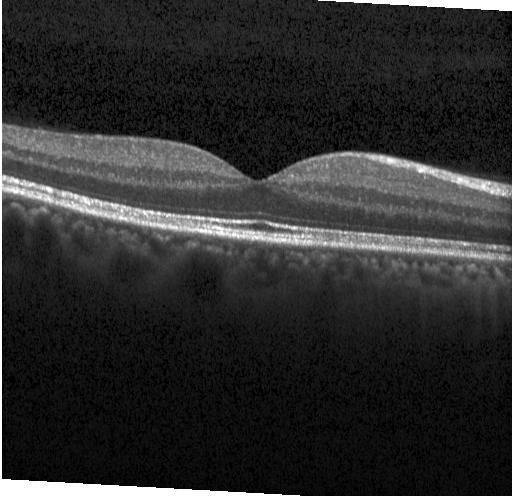
Retinal OCT B-scan. Finding: no choroidal neovascularization, diabetic macular edema, or drusen.